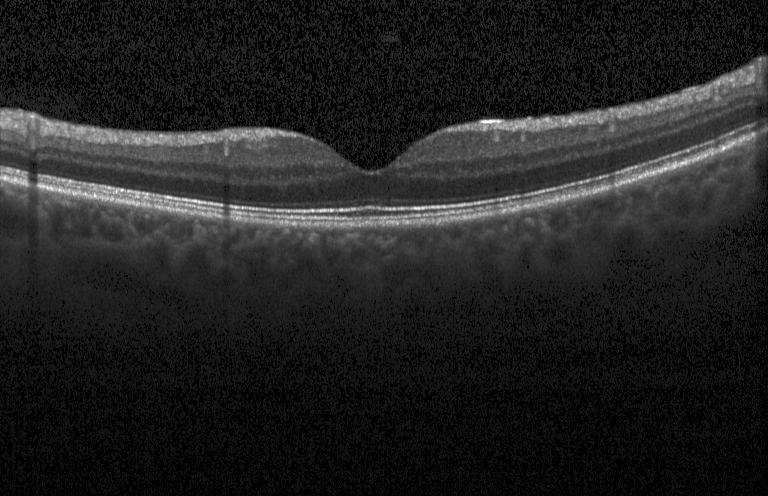
SD-OCT; OCT line scan; fovea-centered; Heidelberg Spectralis — The scan shows no choroidal neovascularization, diabetic macular edema, or drusen.